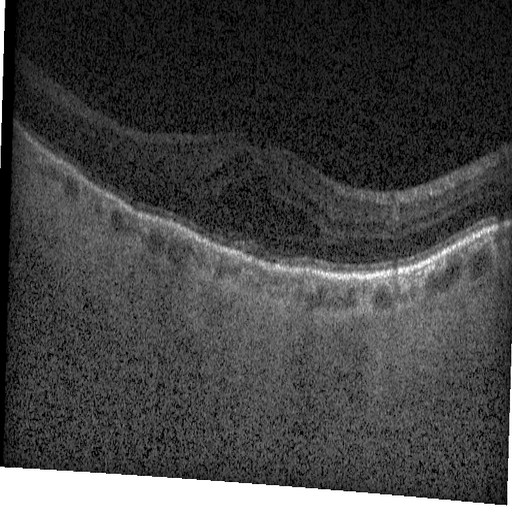 Spectral-domain OCT B-scan: diabetic macular edema.